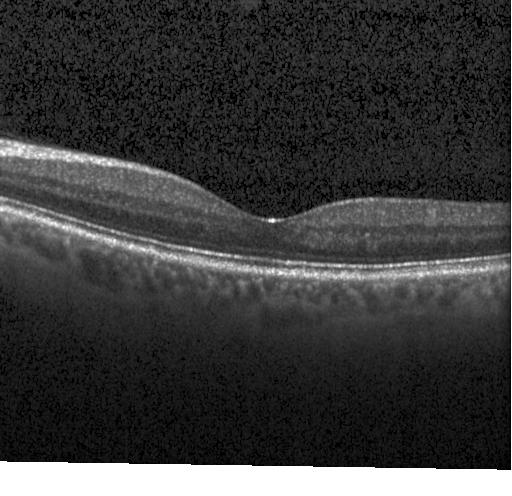
OCT finding: no evidence of CNV, DME, or drusen.